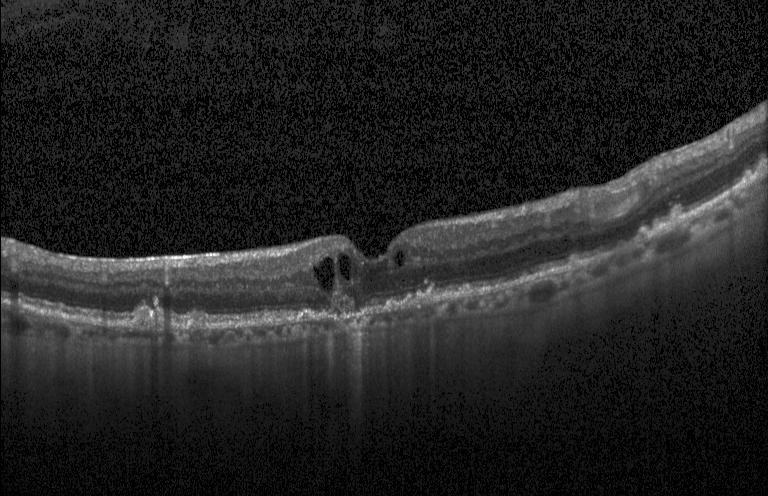 Dx: a choroidal neovascular membrane.